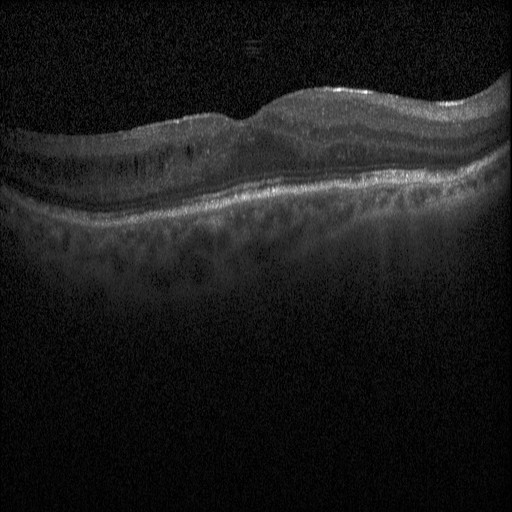

Assessment: diabetic macular edema (DME).